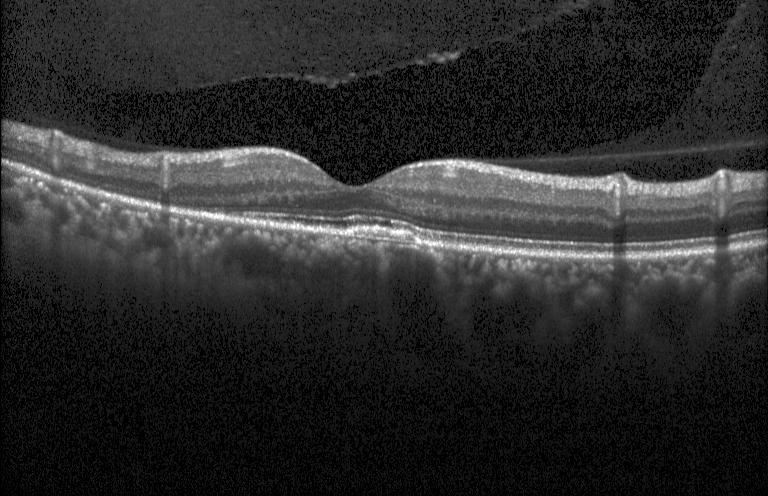

Heidelberg Spectralis OCT system · retinal OCT B-scan — Diagnosis: a choroidal neovascular membrane.